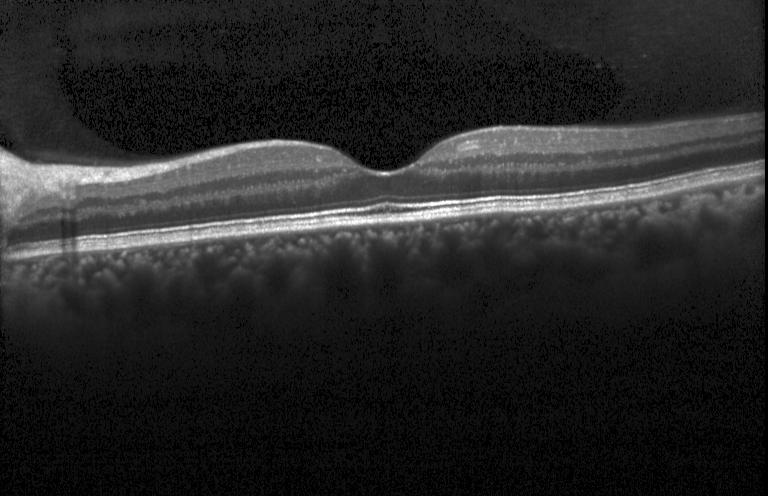

Optical coherence tomography scan. Through the macula. Heidelberg Spectralis OCT system.
Macular OCT: no evidence of CNV, DME, or drusen.